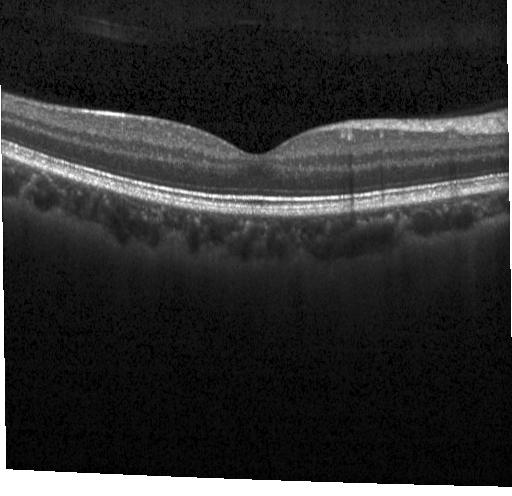

Optical coherence tomography scan.
No evidence of choroidal neovascularization, diabetic macular edema, or drusen.